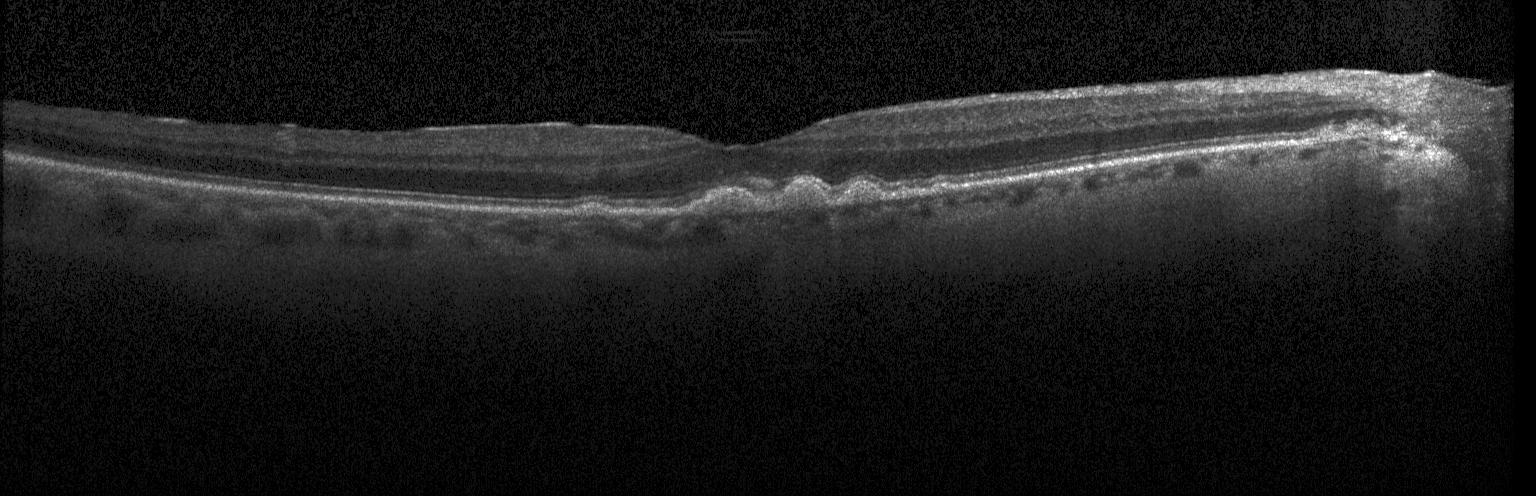
Optical coherence tomography B-scan · spectral-domain OCT — This B-scan demonstrates sub-RPE drusenoid deposits.